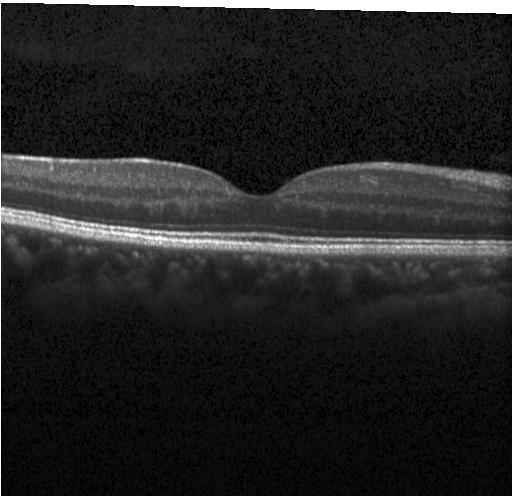 Centered on the fovea. Spectral-domain optical coherence tomography. Optical coherence tomography B-scan.
Finding: no choroidal neovascularization, diabetic macular edema, or drusen.